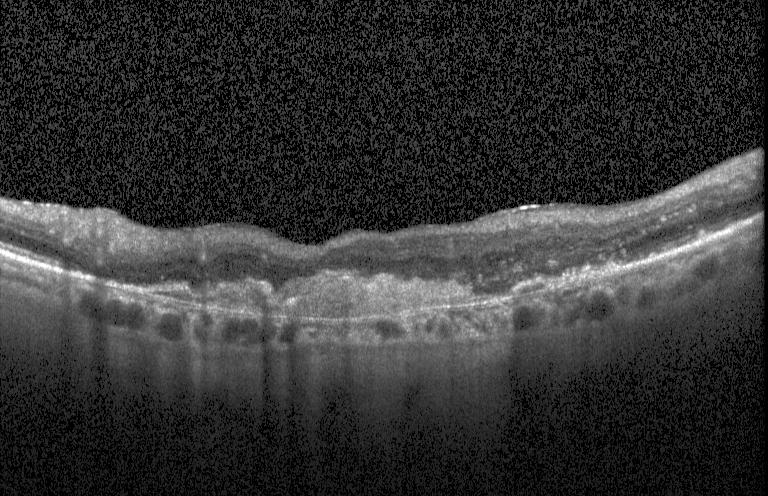

Spectral-domain optical coherence tomography. Fovea-centered. Optical coherence tomography scan. Heidelberg Spectralis OCT system.
Diagnosis: choroidal neovascularization.